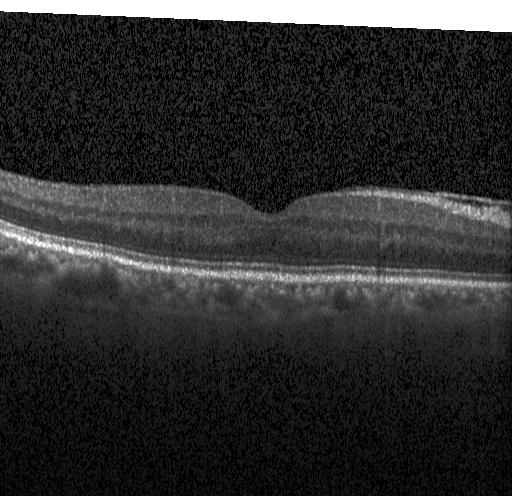
Finding: no evidence of choroidal neovascularization, diabetic macular edema, or drusen.